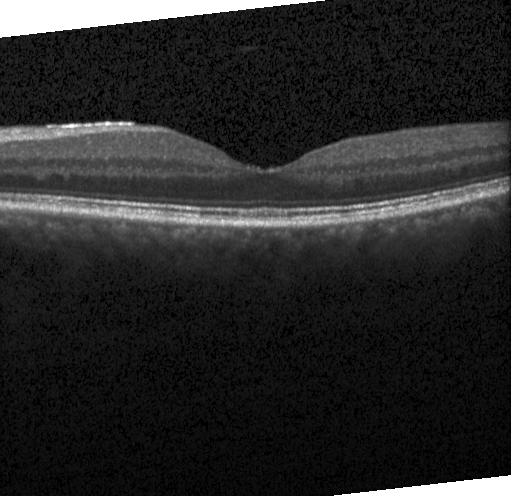
Optical coherence tomography scan · through the macula · acquired on a Heidelberg Spectralis · SD-OCT — Finding: no CNV, no DME, and no drusen.